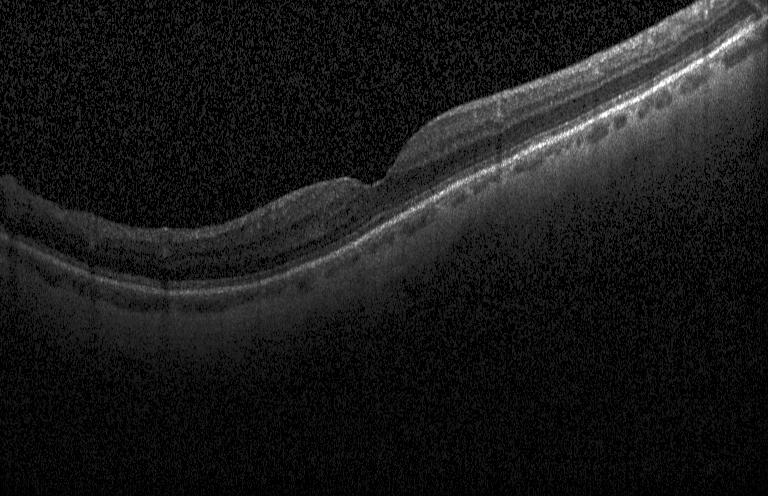 Impression: neither choroidal neovascularization, diabetic macular edema, nor drusen.